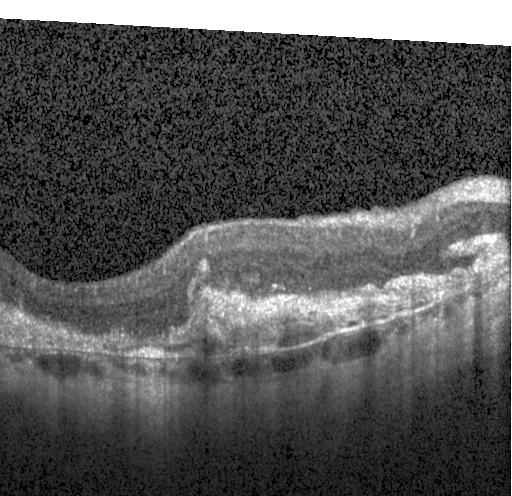
Centered on the fovea; retinal OCT B-scan; Heidelberg Spectralis. Diagnosis: choroidal neovascularization (CNV).